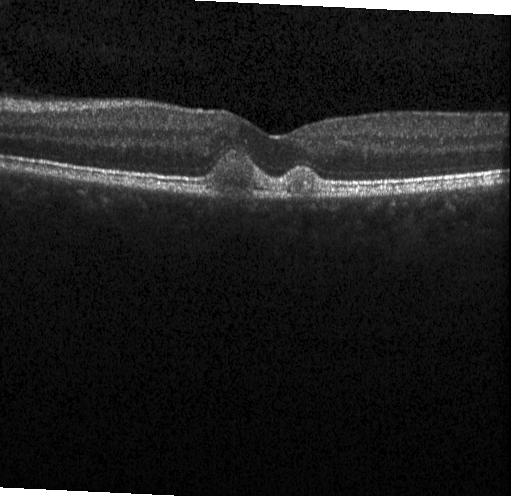

Optical coherence tomography B-scan
Assessment: sub-RPE drusenoid deposits.